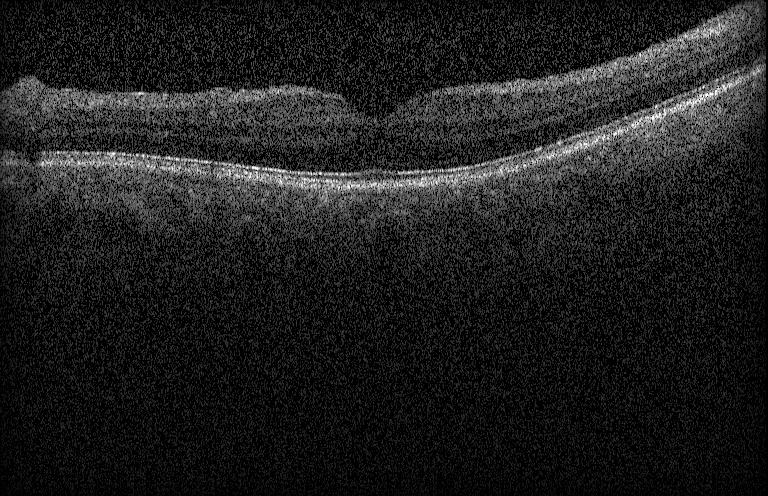 Fovea-centered. Spectral-domain OCT. Heidelberg Spectralis OCT system. OCT line scan — Assessment: no CNV, DME, or drusen.